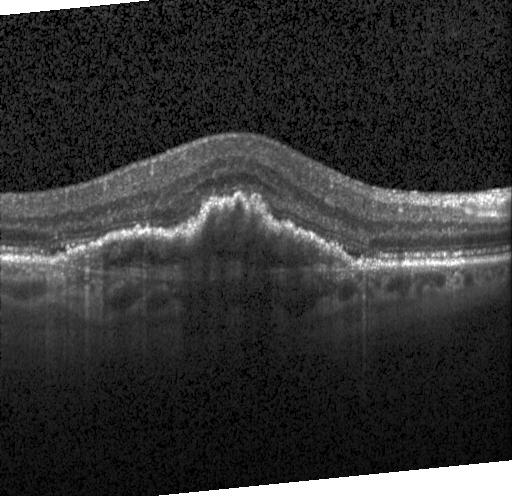

Retinal OCT B-scan.
Diagnosis: a choroidal neovascular membrane.